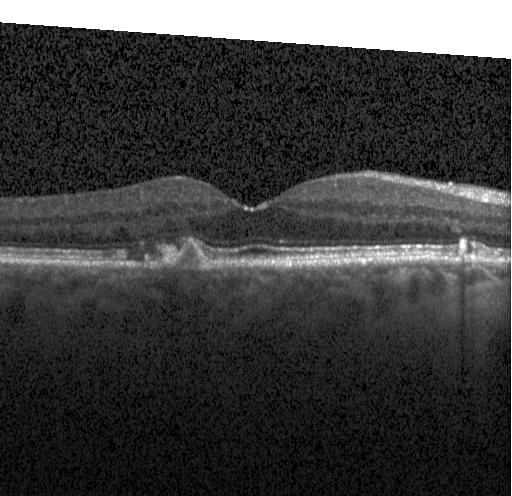

This B-scan demonstrates choroidal neovascularization (CNV).